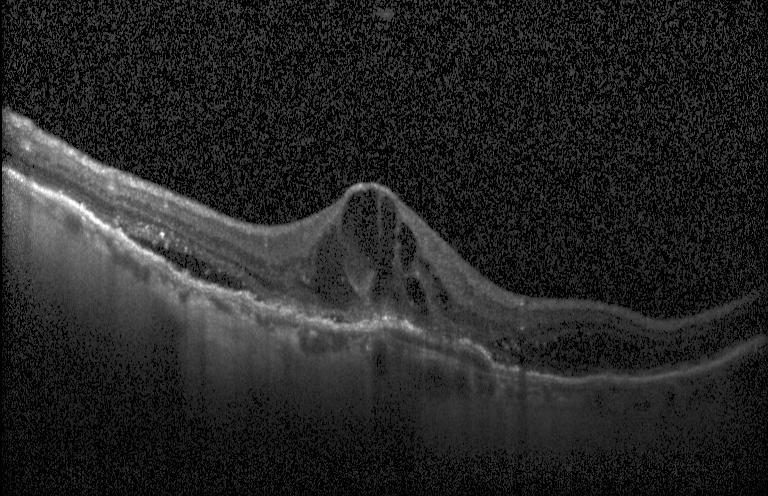
Spectral-domain OCT B-scan: choroidal neovascularization.